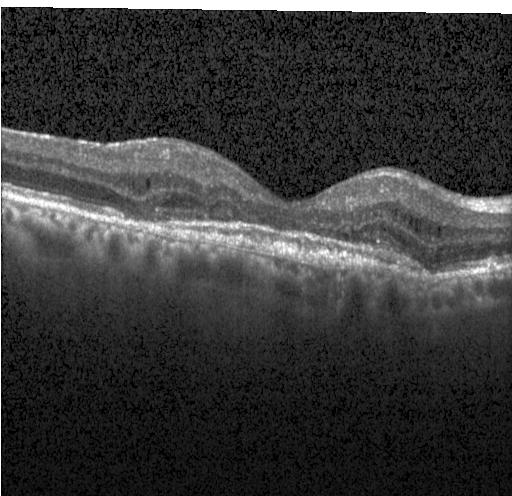 Impression: choroidal neovascularization.